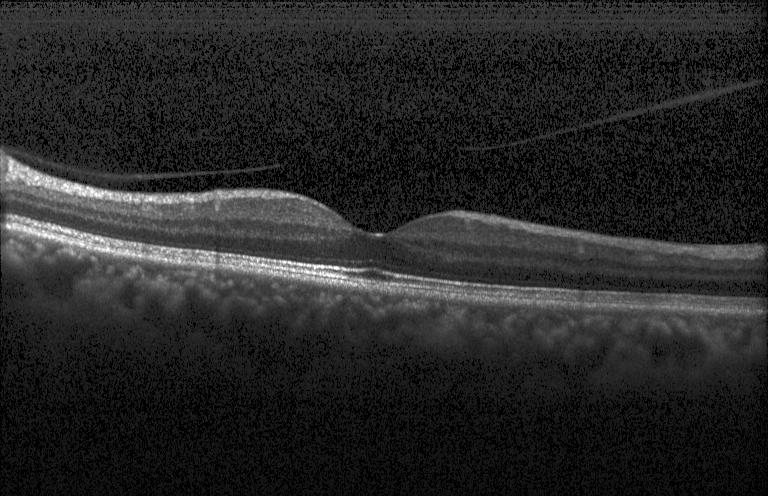 OCT line scan · instrument: Heidelberg Spectralis · SD-OCT — The scan shows no CNV, DME, or drusen.